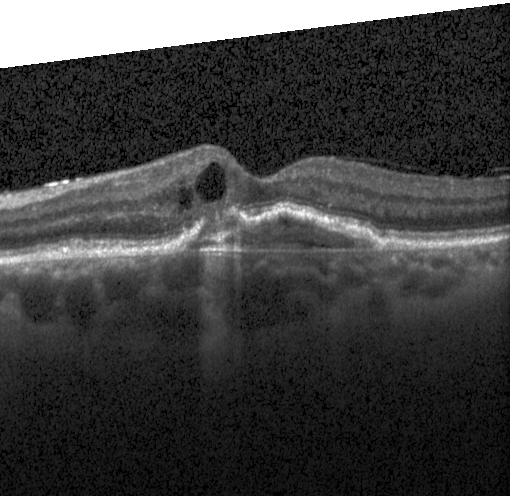 OCT line scan.
This B-scan demonstrates CNV.